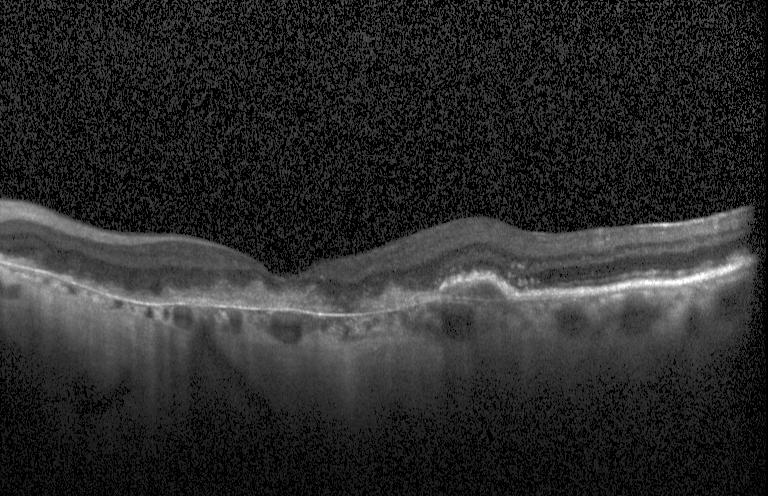 Optical coherence tomography scan; through the macula
CNV.